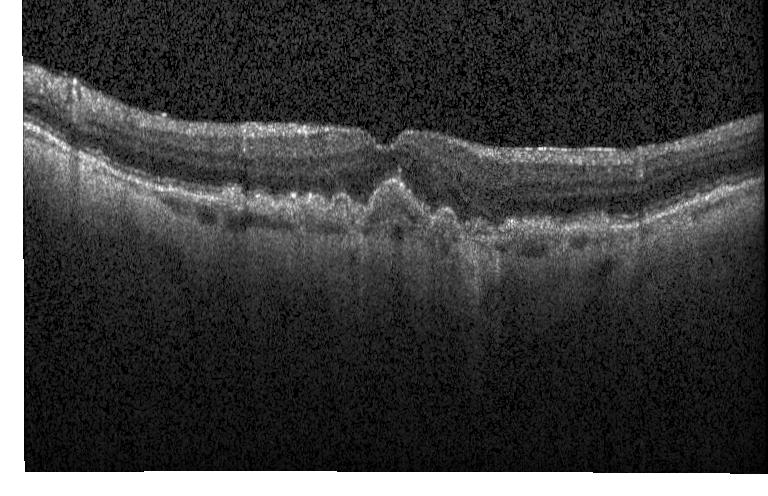 Spectral-domain OCT B-scan: a choroidal neovascular membrane.